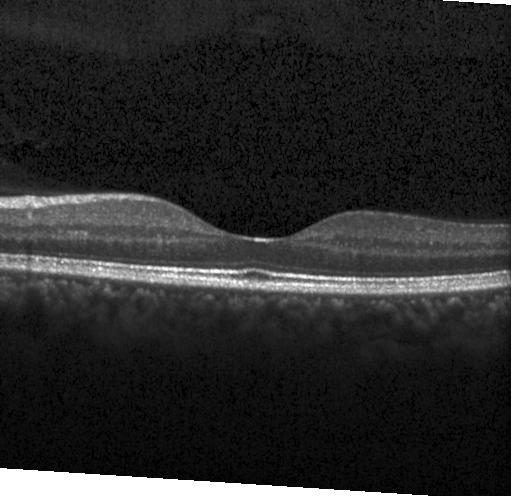 Heidelberg Spectralis OCT system · retinal OCT B-scan
Neither choroidal neovascularization, diabetic macular edema, nor drusen.